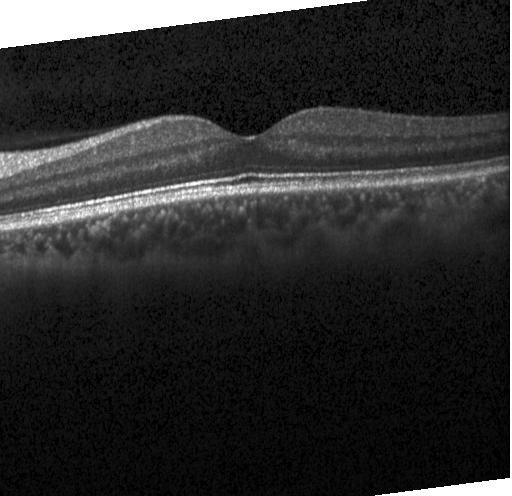 Dx: no choroidal neovascularization, diabetic macular edema, or drusen.